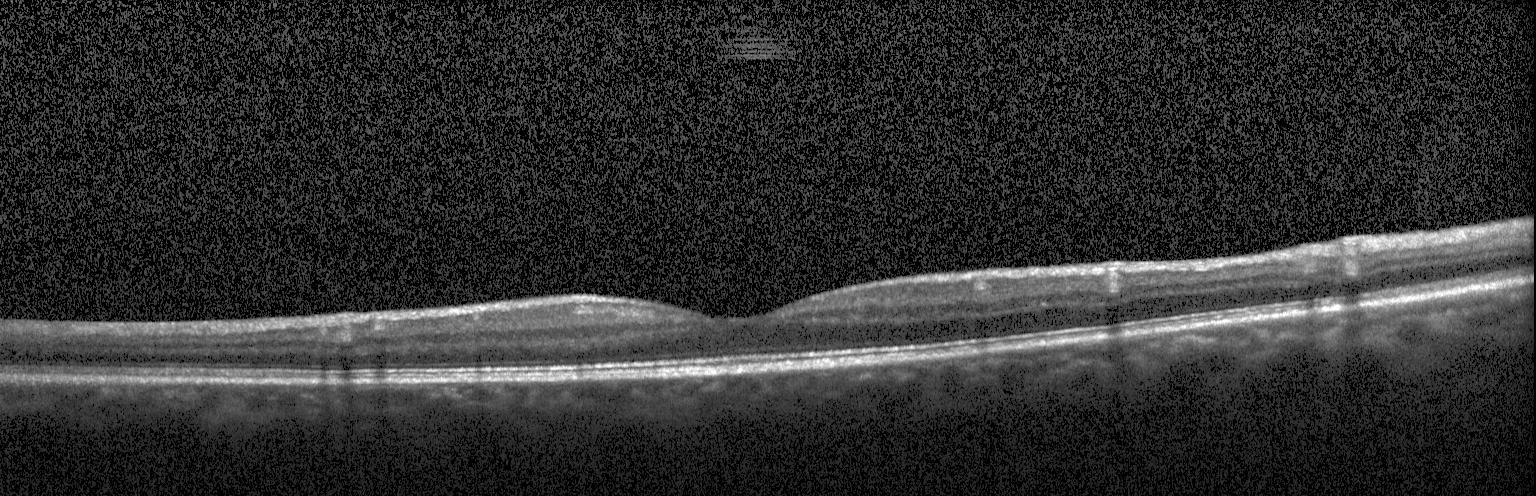

This B-scan demonstrates no evidence of choroidal neovascularization, diabetic macular edema, or drusen.